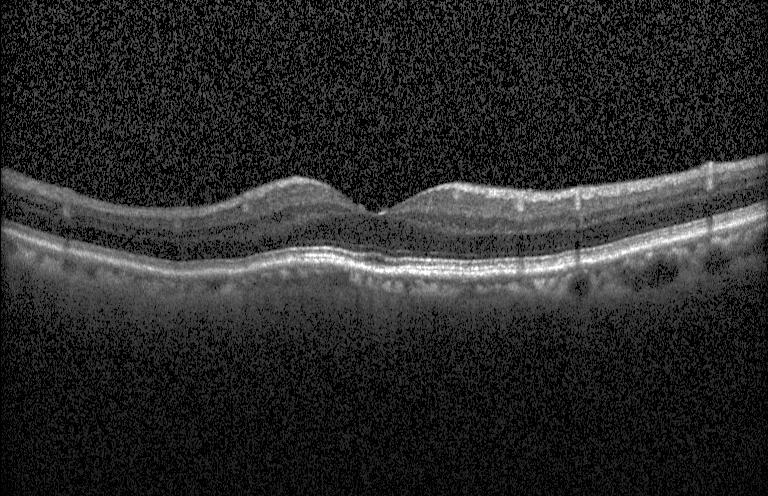
OCT line scan.
Finding: no choroidal neovascularization, no diabetic macular edema, and no drusen.